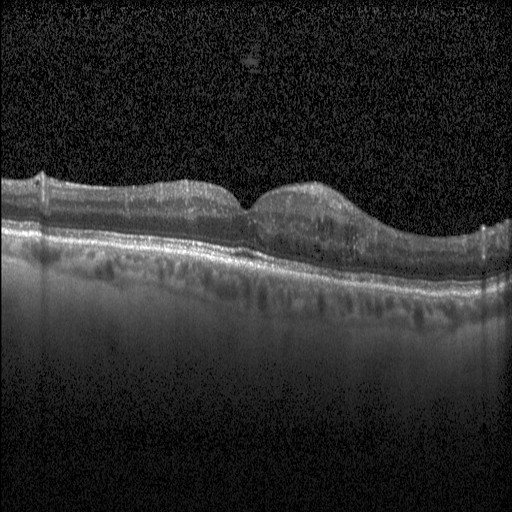
Finding: DME.